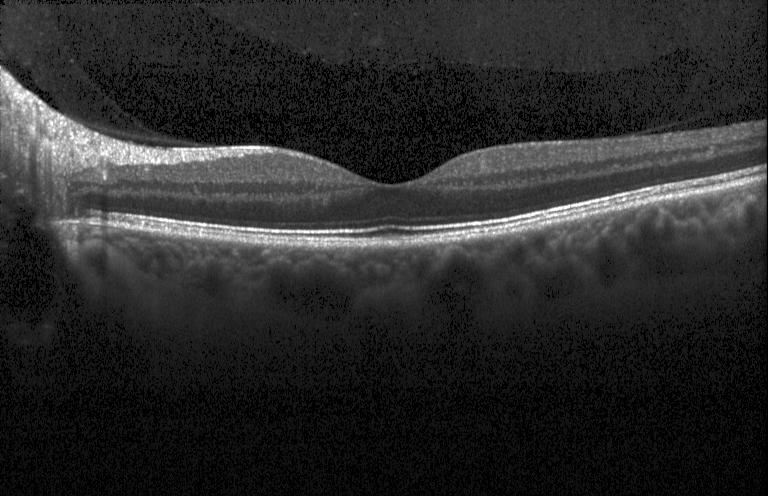 No choroidal neovascularization, no diabetic macular edema, and no drusen.